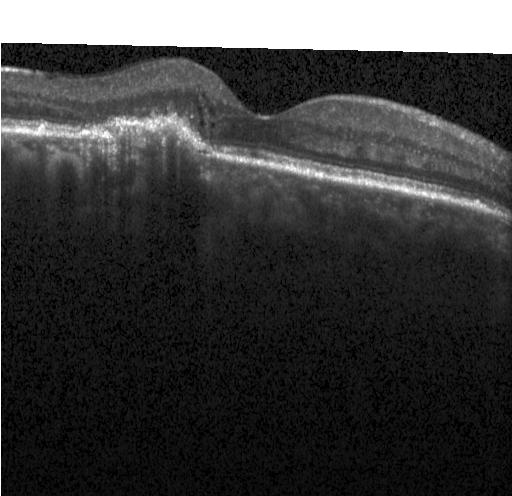

Retinal OCT B-scan. OCT finding: a choroidal neovascular membrane.